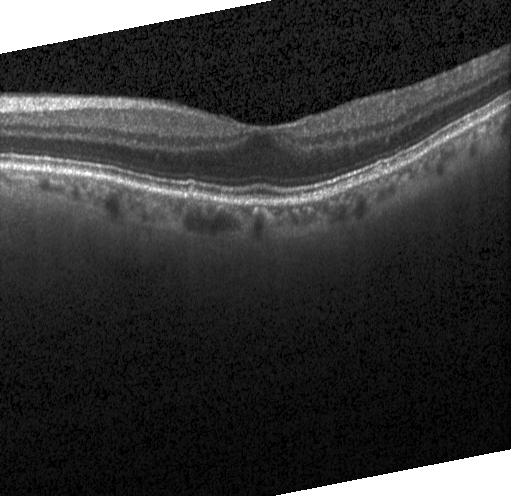

Impression: drusen.